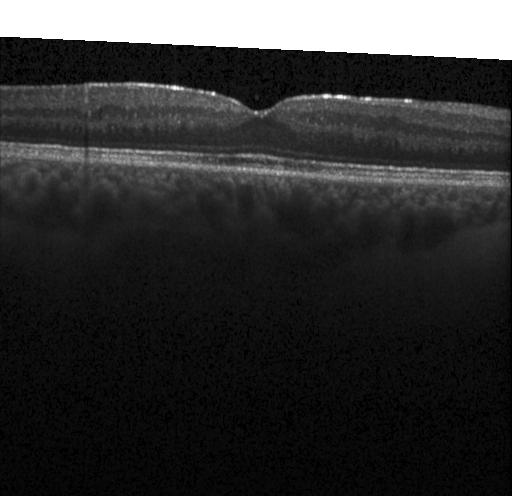

Optical coherence tomography B-scan, through the macula, spectral-domain optical coherence tomography.
Finding: no choroidal neovascularization, no diabetic macular edema, and no drusen.